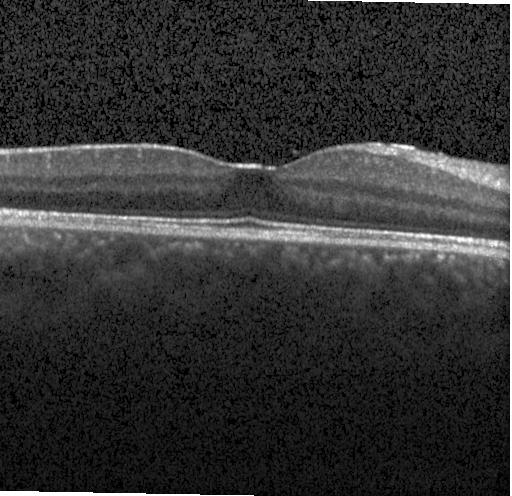
The scan shows no choroidal neovascularization, diabetic macular edema, or drusen.